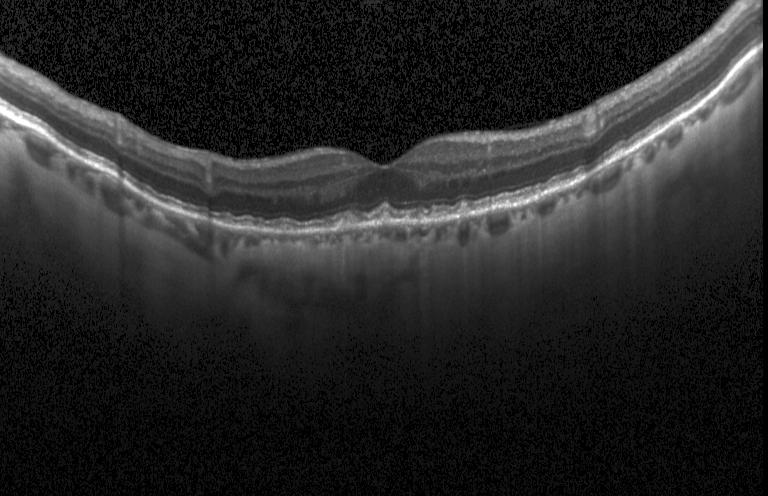 SD-OCT. OCT B-scan. Drusen.